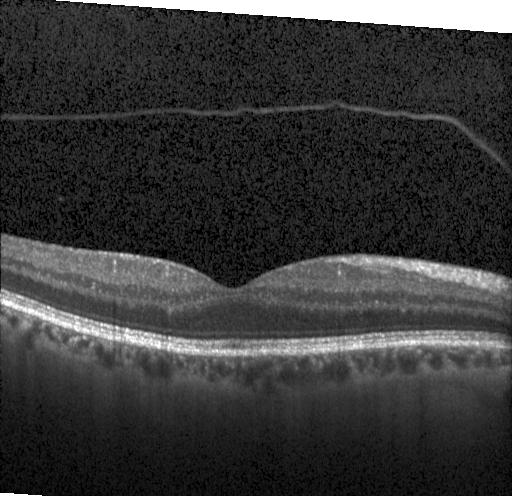
Optical coherence tomography B-scan. Through the macula — Macular OCT: no CNV, no DME, and no drusen.